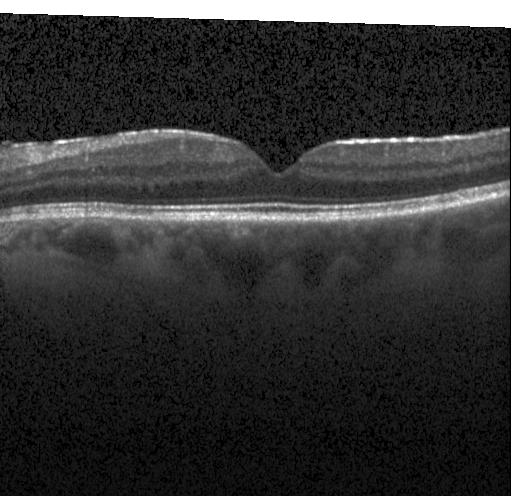 Through the macula, optical coherence tomography scan, spectral-domain optical coherence tomography
Dx: no choroidal neovascularization, no diabetic macular edema, and no drusen.